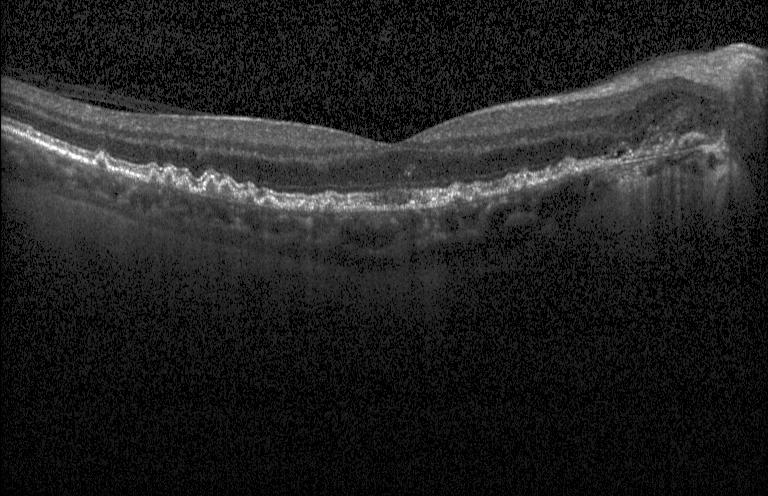 Retinal OCT cross-section showing a choroidal neovascular membrane.